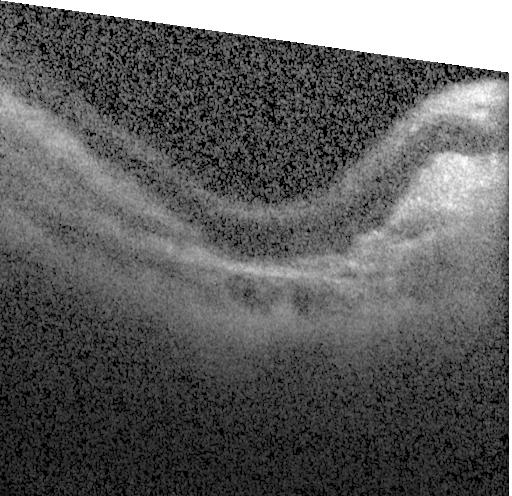 Spectral-domain optical coherence tomography, instrument: Heidelberg Spectralis, fovea-centered, OCT line scan
Diagnosis: a choroidal neovascular membrane.